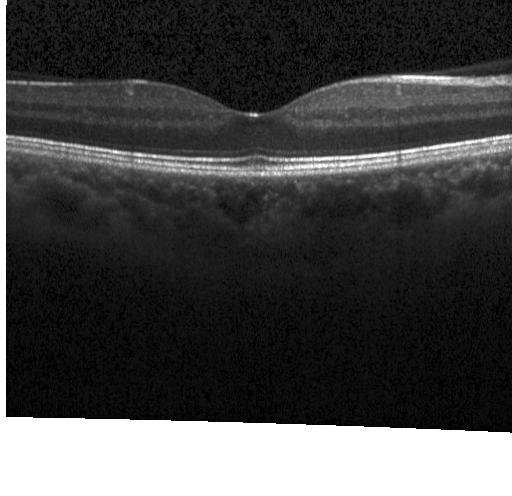

OCT B-scan showing neither choroidal neovascularization, diabetic macular edema, nor drusen.